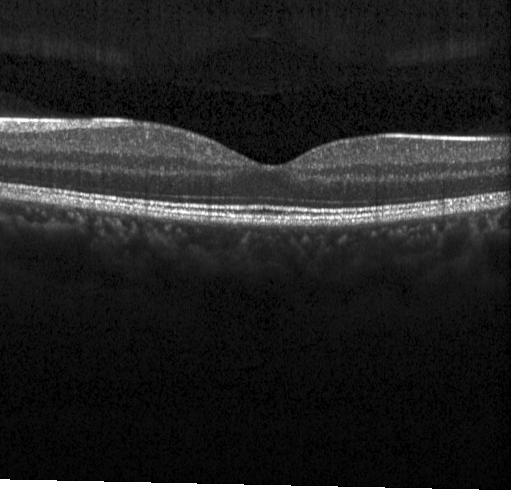

Spectral-domain optical coherence tomography, retinal OCT cross-section, centered on the fovea, acquired on a Heidelberg Spectralis — Finding: neither CNV, DME, nor drusen.